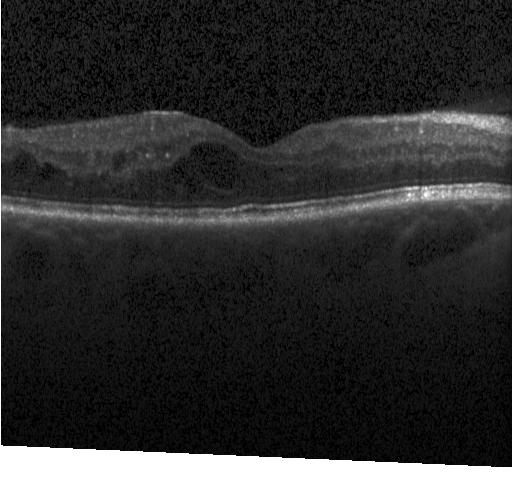 OCT finding: diabetic macular edema (DME).